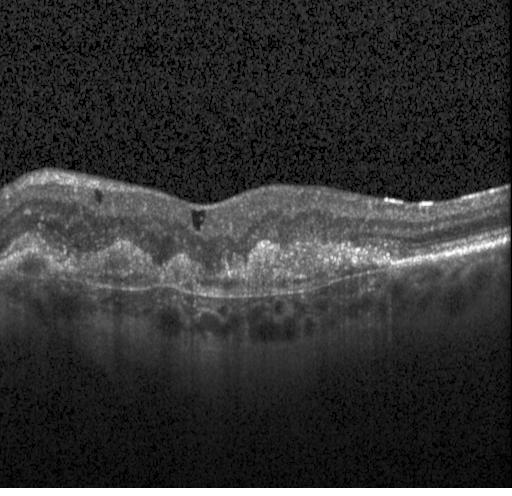 Spectral-domain OCT B-scan: a choroidal neovascular membrane.